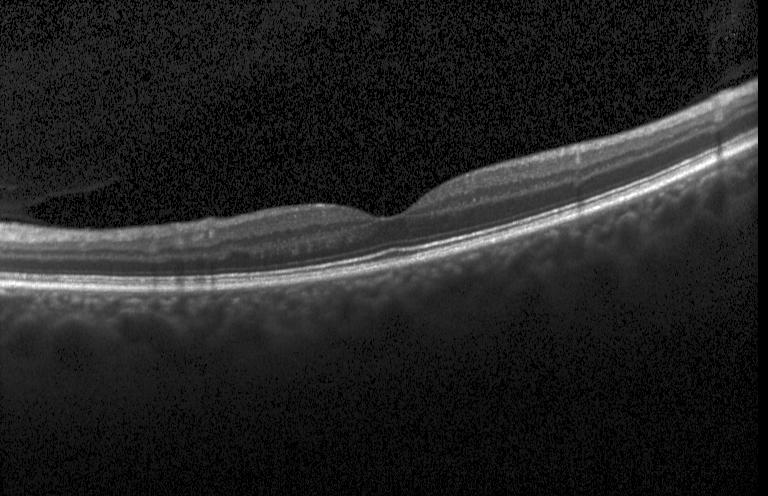
Instrument: Heidelberg Spectralis, retinal OCT cross-section
No choroidal neovascularization, diabetic macular edema, or drusen.